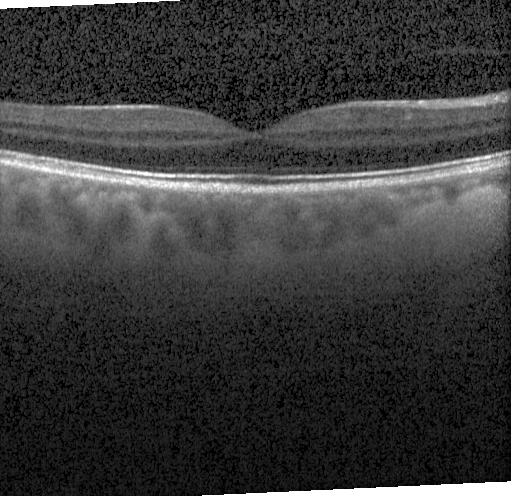
OCT B-scan · SD-OCT · acquired on a Heidelberg Spectralis
Impression: neither choroidal neovascularization, diabetic macular edema, nor drusen.